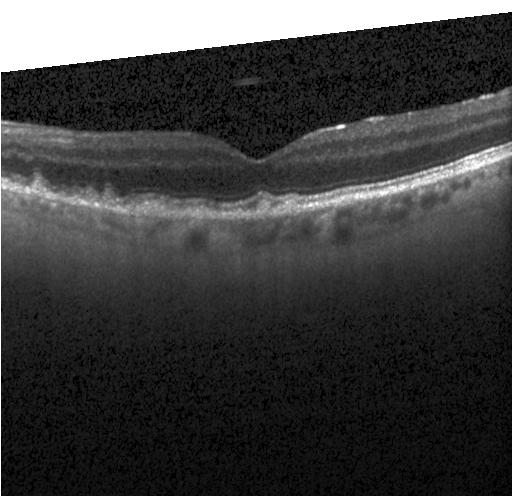

OCT B-scan showing drusen.